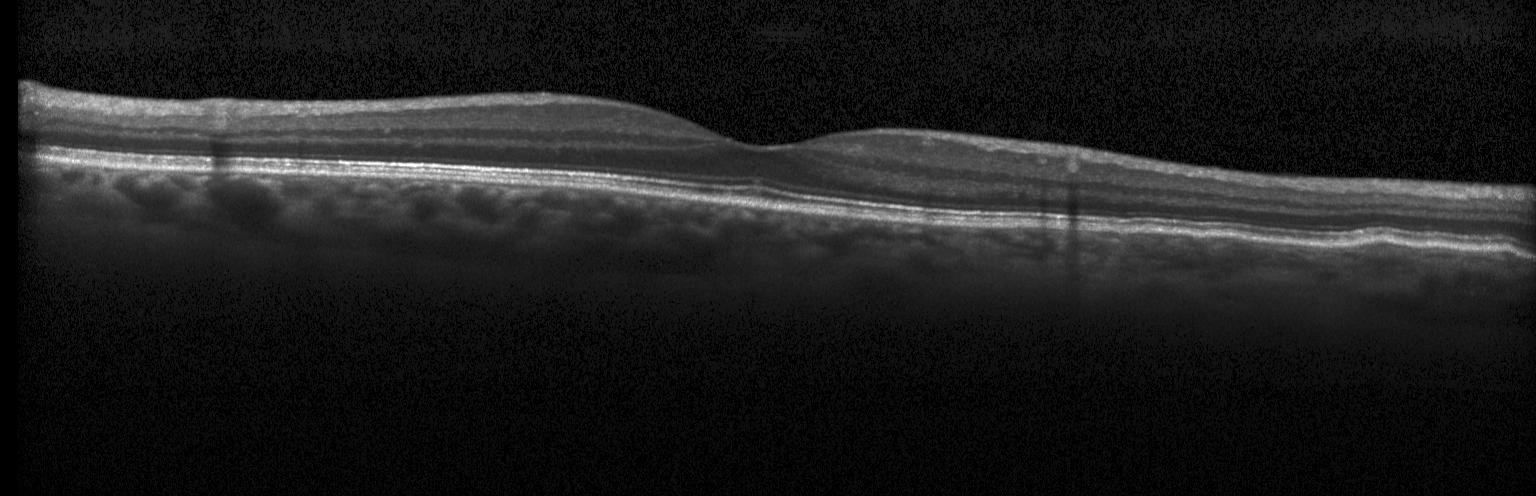

OCT finding: no choroidal neovascularization, no diabetic macular edema, and no drusen.